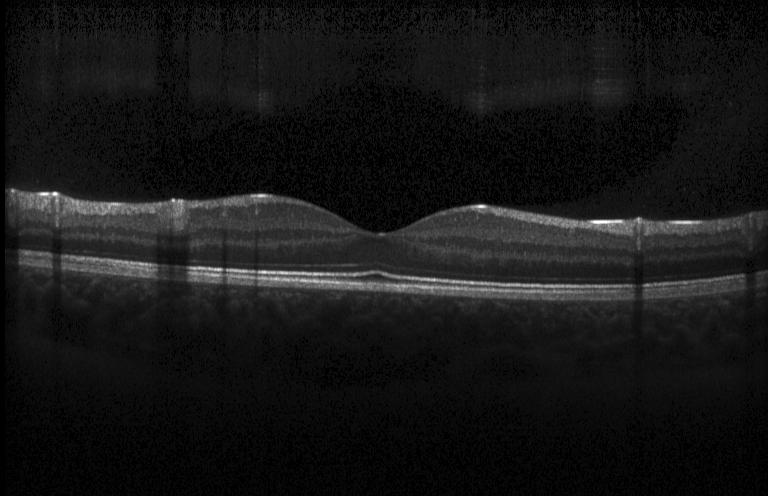 Macular OCT demonstrating no choroidal neovascularization, diabetic macular edema, or drusen.